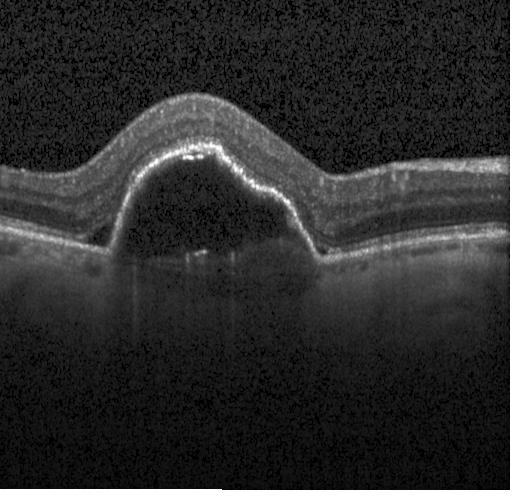 Macular OCT: choroidal neovascularization (CNV).